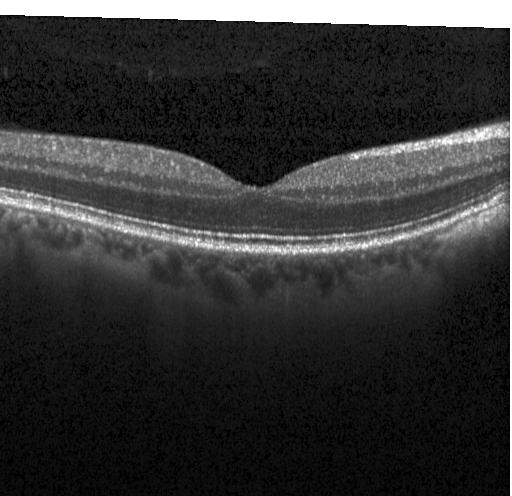
Impression: no evidence of choroidal neovascularization, diabetic macular edema, or drusen.